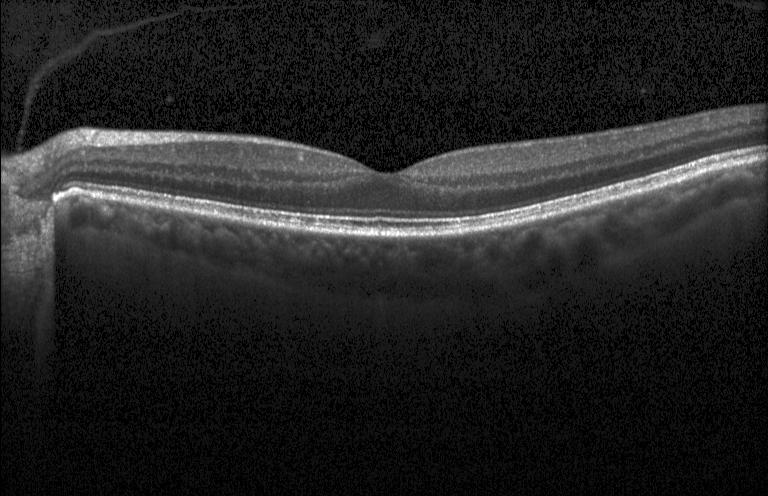

Retinal OCT cross-section. Diagnosis: neither choroidal neovascularization, diabetic macular edema, nor drusen.